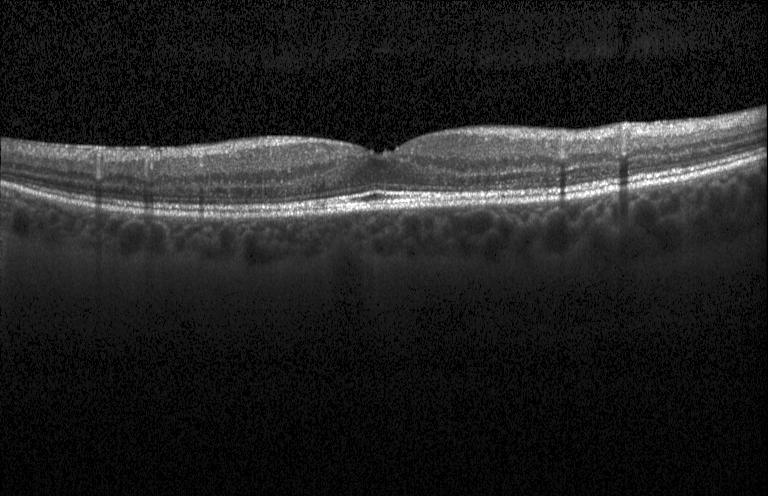

Through the macula; optical coherence tomography scan; instrument: Heidelberg Spectralis.
The scan shows no choroidal neovascularization, no diabetic macular edema, and no drusen.